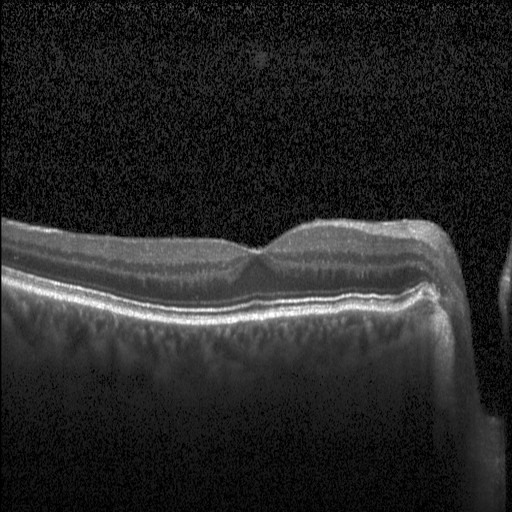
Dx: DME.